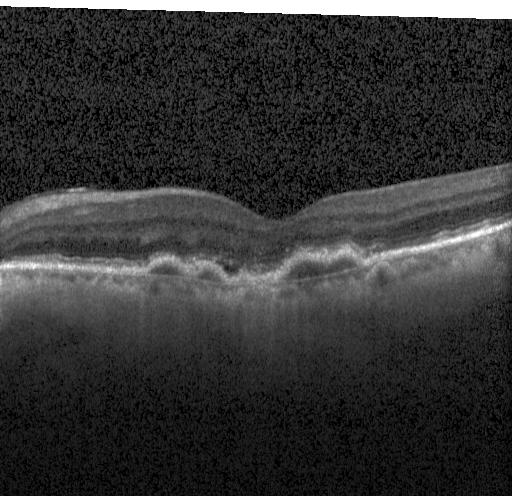 Impression: a choroidal neovascular membrane.